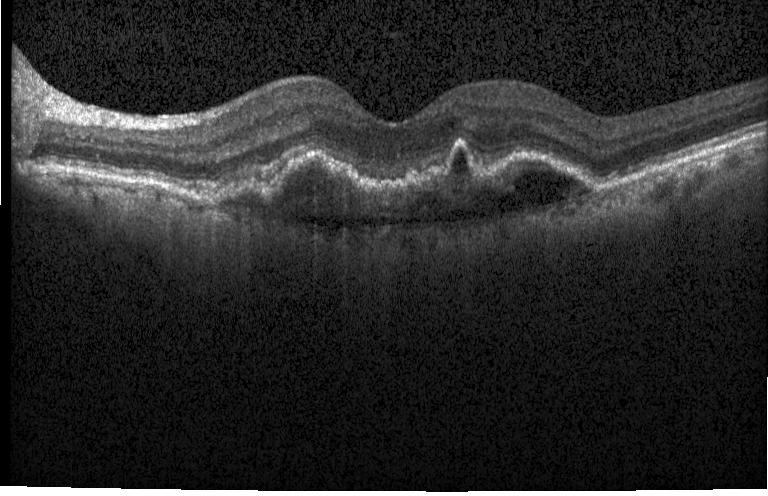

Assessment: a choroidal neovascular membrane.